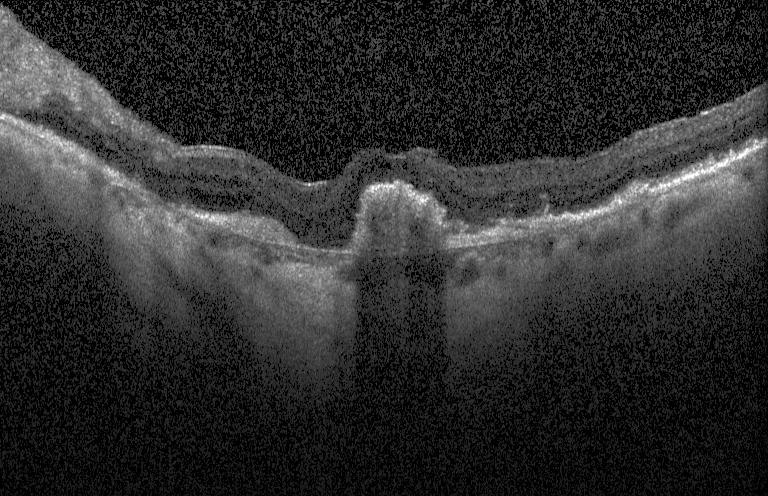 Macular OCT demonstrating choroidal neovascularization (CNV).